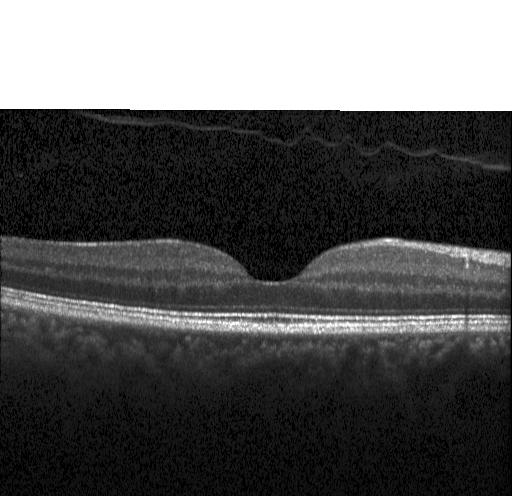

The scan shows neither choroidal neovascularization, diabetic macular edema, nor drusen.